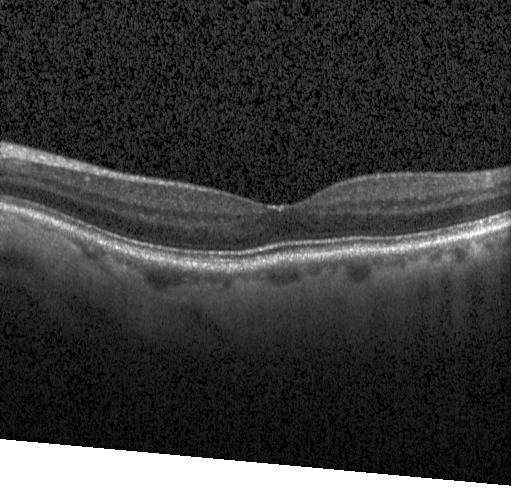 OCT B-scan · through the macula
Diagnosis: no choroidal neovascularization, diabetic macular edema, or drusen.